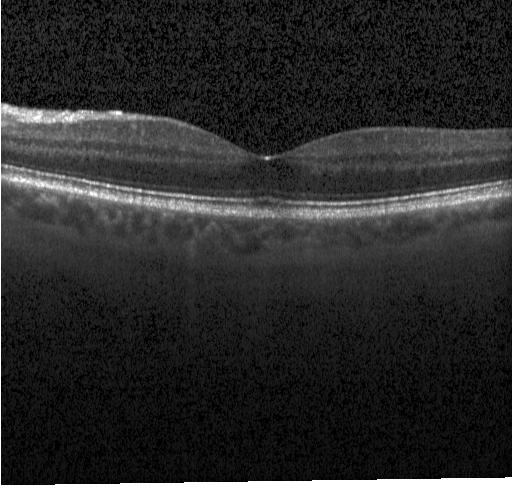 Centered on the fovea; retinal OCT cross-section; acquired on a Heidelberg Spectralis; spectral-domain optical coherence tomography
Macular OCT: no evidence of CNV, DME, or drusen.